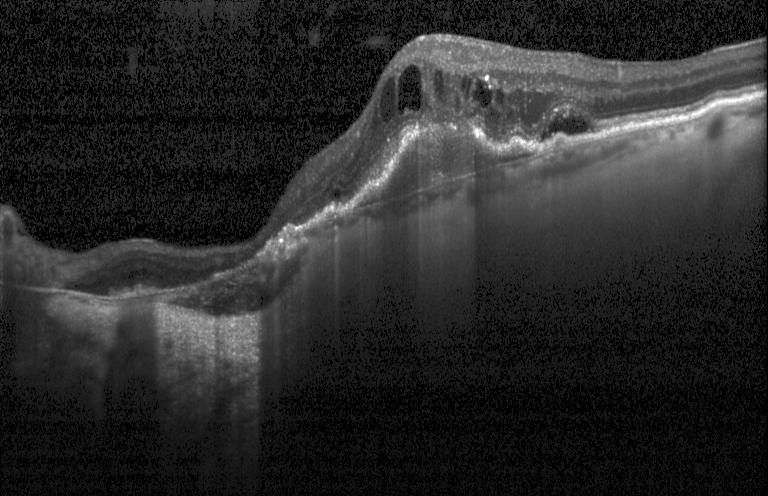

SD-OCT, retinal OCT cross-section.
The scan shows CNV.